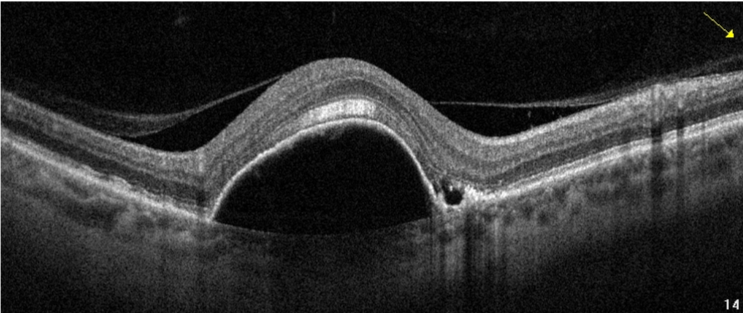 Through the macula. Acquired on an Optovue Avanti RTVue XR. Optical coherence tomography B-scan — Impression: age-related macular degeneration.